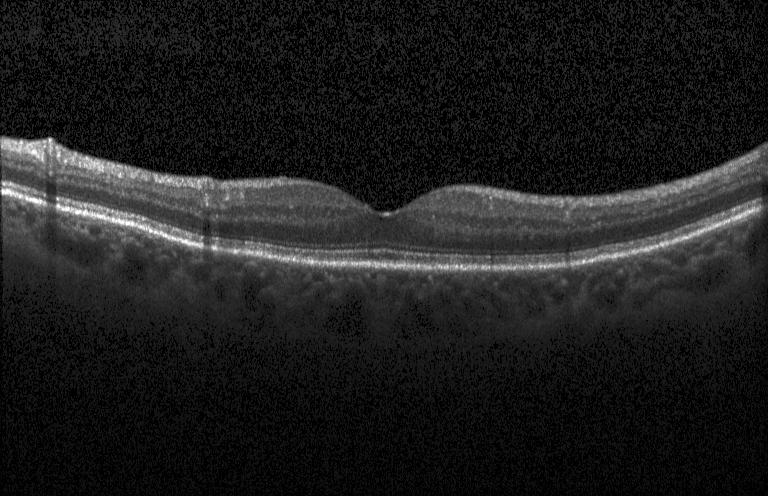
Retinal OCT B-scan.
The scan shows neither choroidal neovascularization, diabetic macular edema, nor drusen.